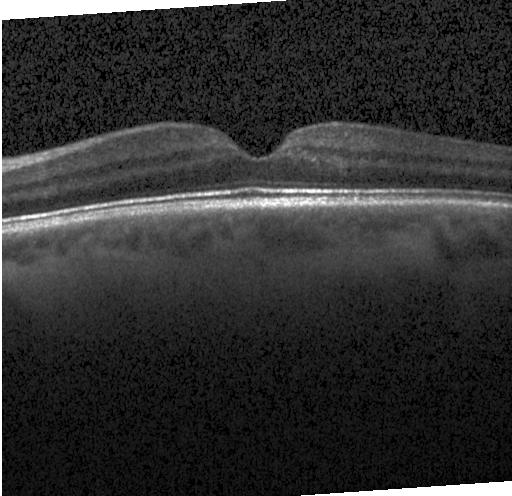
Optical coherence tomography B-scan. Macular OCT: no evidence of choroidal neovascularization, diabetic macular edema, or drusen.